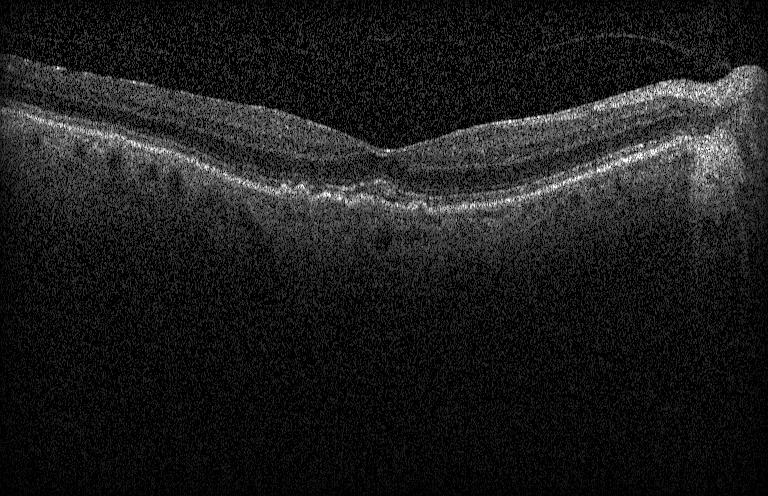
OCT B-scan, spectral-domain optical coherence tomography.
Assessment: a choroidal neovascular membrane.